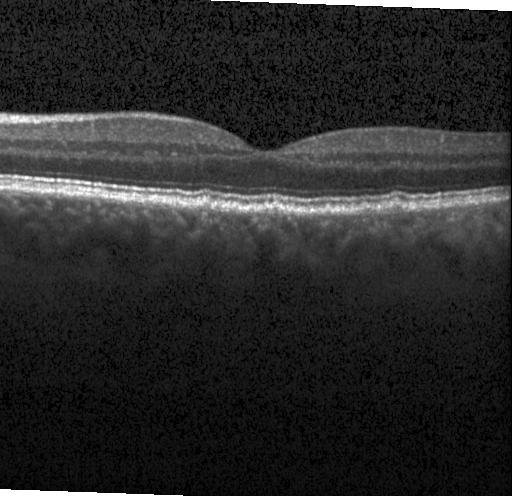 Finding: multiple drusen.